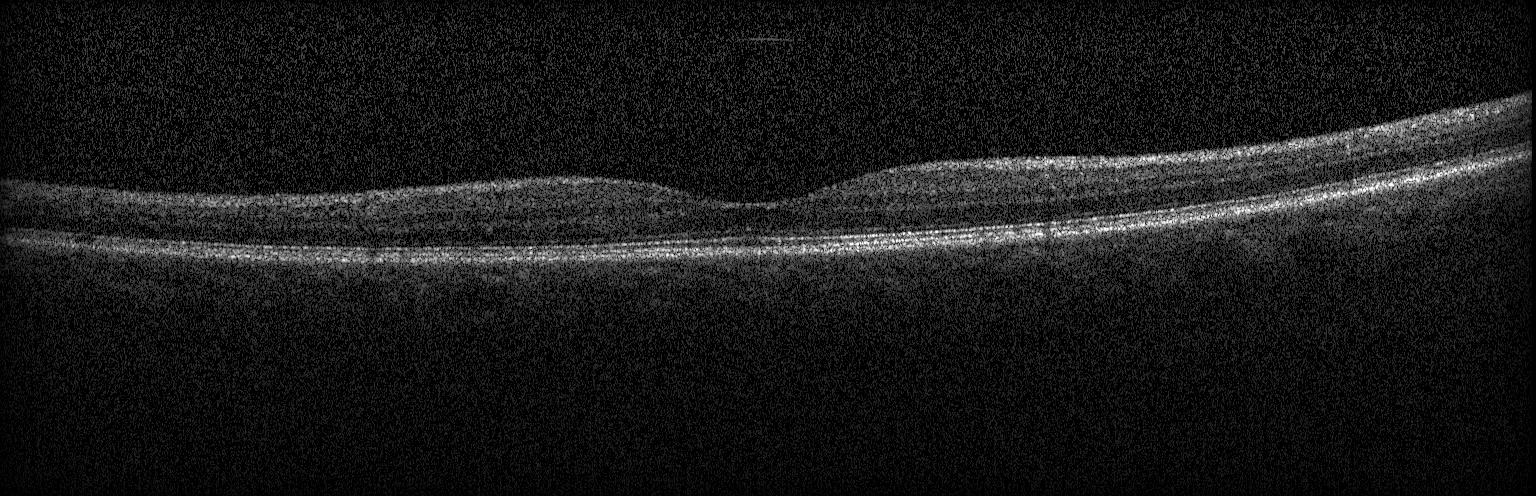 Macular scan; instrument: Heidelberg Spectralis; optical coherence tomography B-scan. Finding: no choroidal neovascularization, no diabetic macular edema, and no drusen.